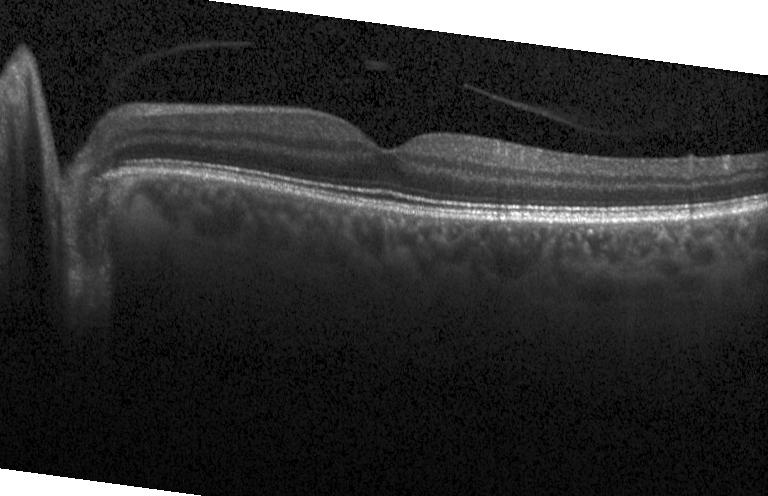 Impression: no choroidal neovascularization, no diabetic macular edema, and no drusen.